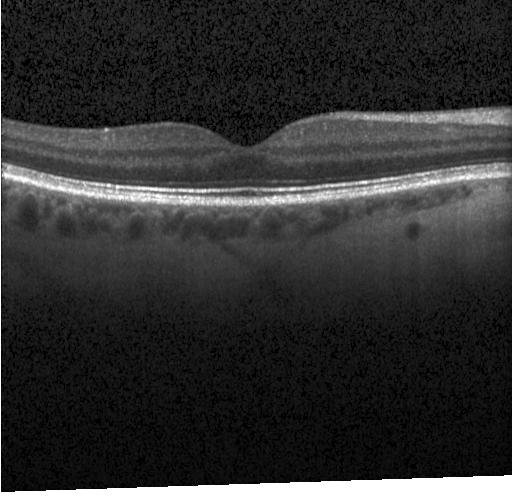 OCT line scan · through the macula. This B-scan demonstrates neither choroidal neovascularization, diabetic macular edema, nor drusen.